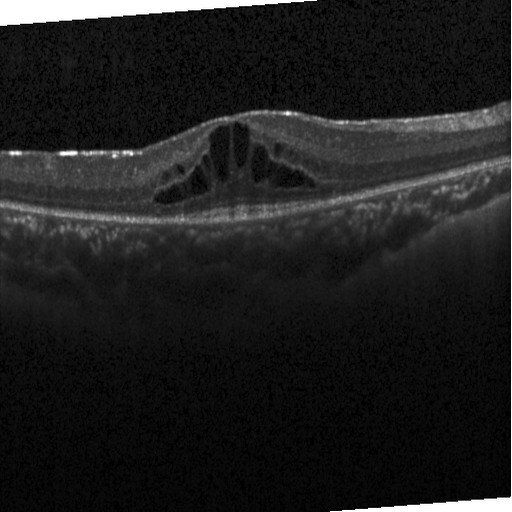 Retinal OCT cross-section showing DME.